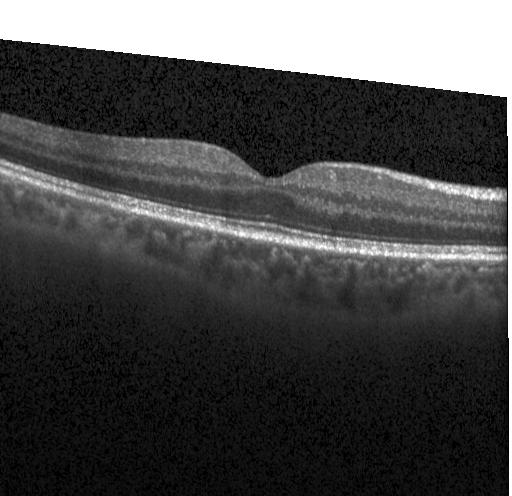
Instrument: Heidelberg Spectralis; fovea-centered; OCT B-scan
Dx: no choroidal neovascularization, no diabetic macular edema, and no drusen.